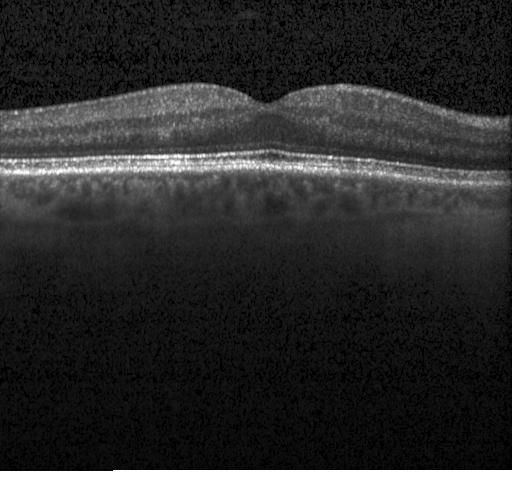
Assessment: no evidence of CNV, DME, or drusen.